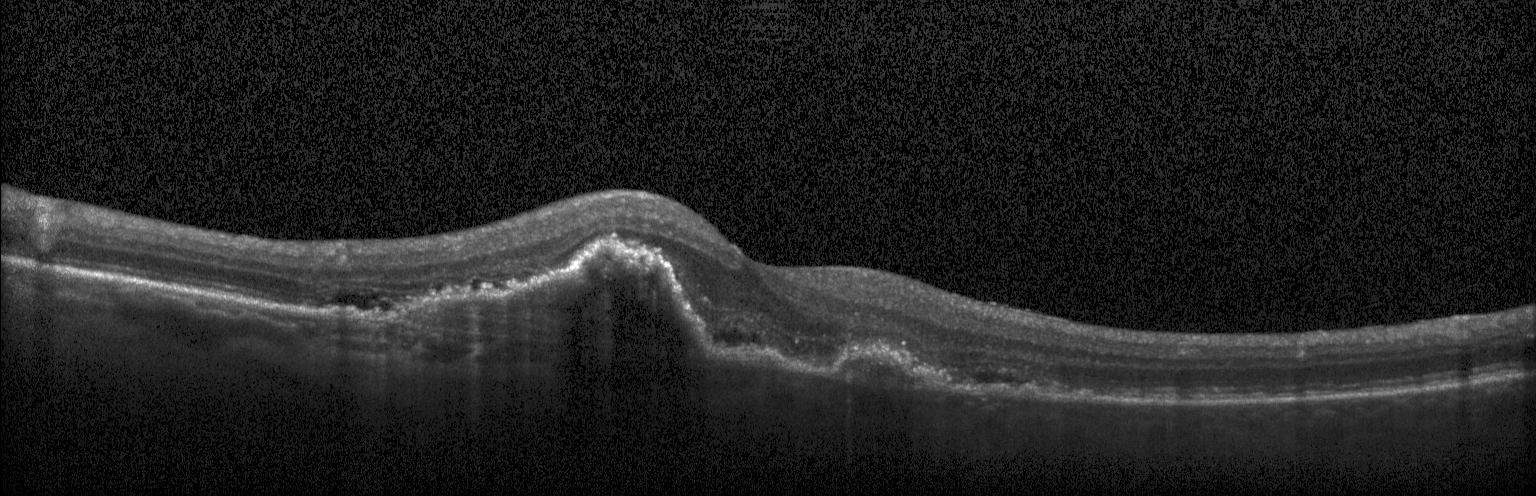

OCT line scan.
Assessment: a choroidal neovascular membrane.